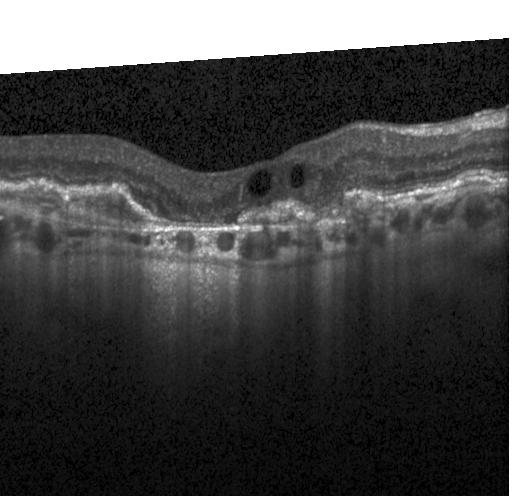
OCT B-scan — Dx: choroidal neovascularization.